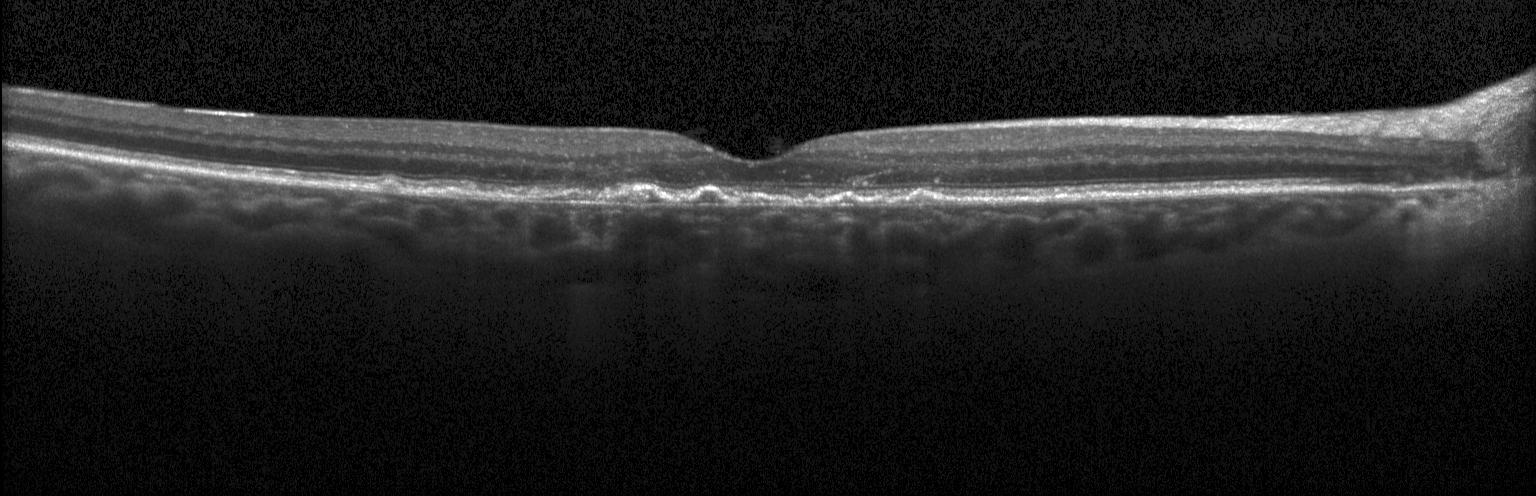

Spectral-domain optical coherence tomography; optical coherence tomography scan; acquired on a Heidelberg Spectralis; fovea-centered
Impression: a choroidal neovascular membrane.